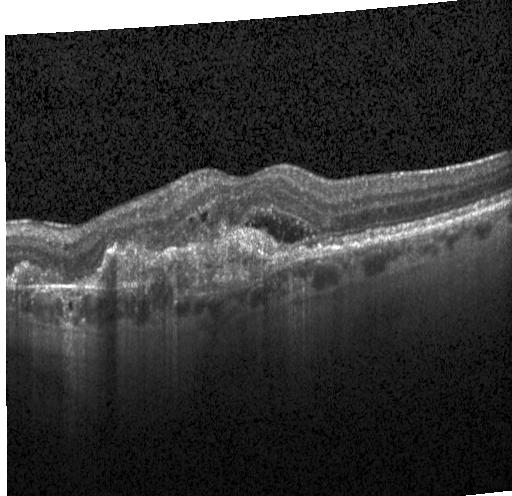
Dx: a choroidal neovascular membrane.